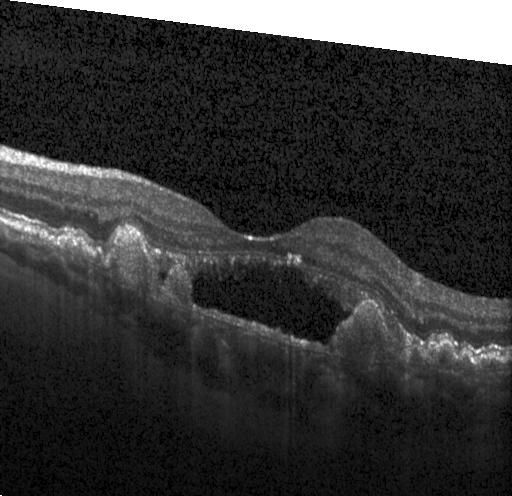
Retinal OCT cross-section showing choroidal neovascularization (CNV).